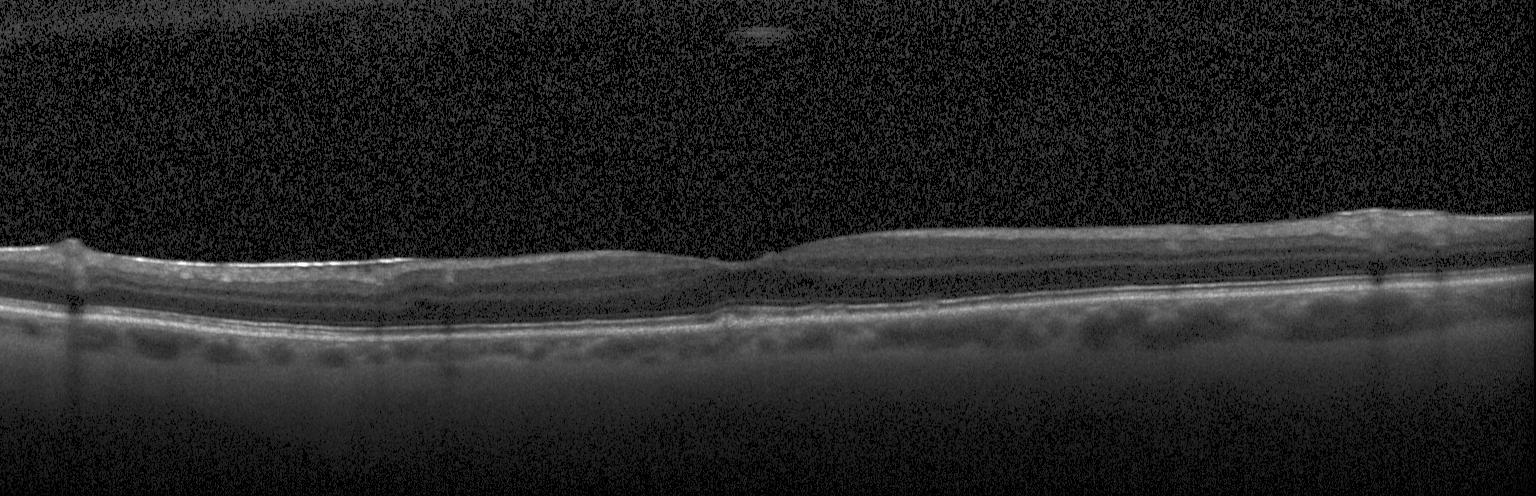

Assessment: multiple drusen.